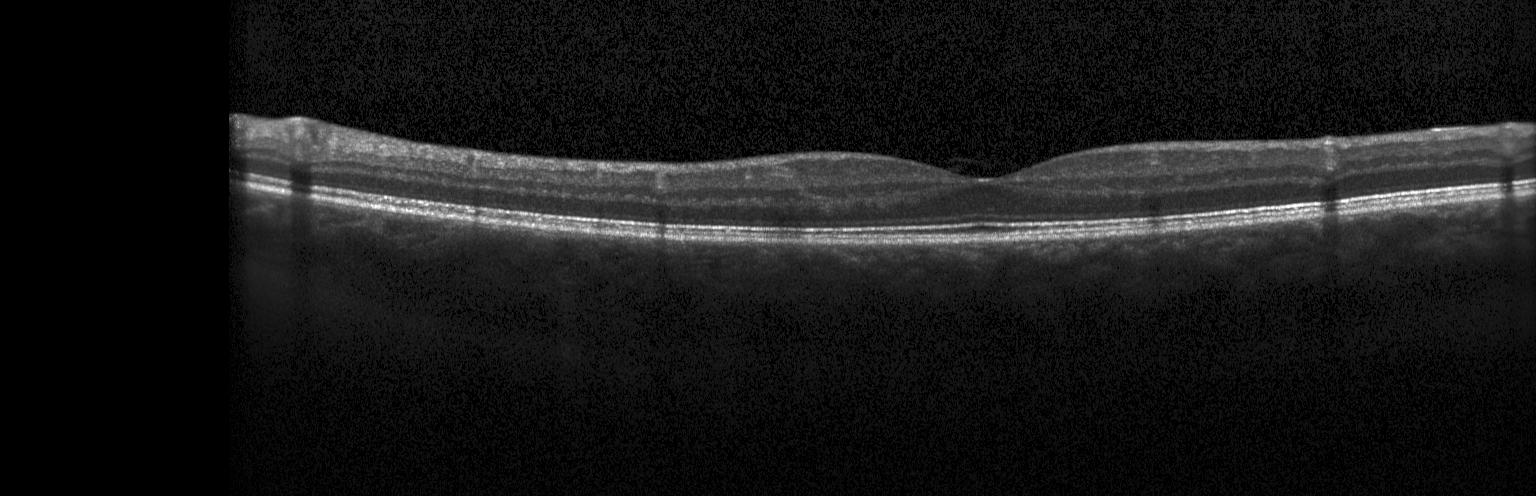 Spectral-domain OCT B-scan: no choroidal neovascularization, no diabetic macular edema, and no drusen.